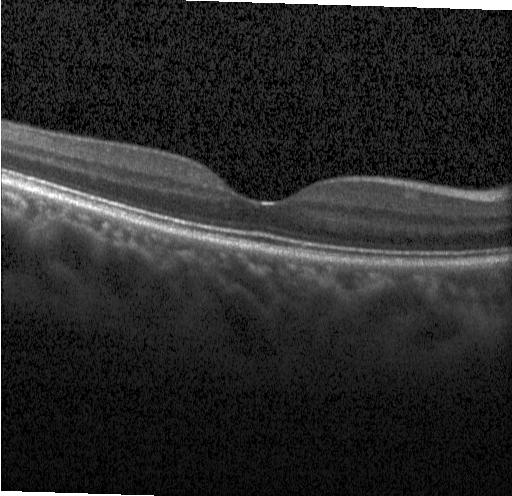

OCT finding: no choroidal neovascularization, no diabetic macular edema, and no drusen.